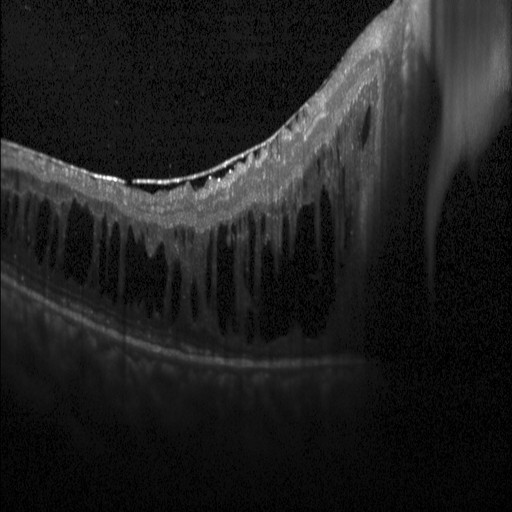

OCT line scan.
This B-scan demonstrates DME.